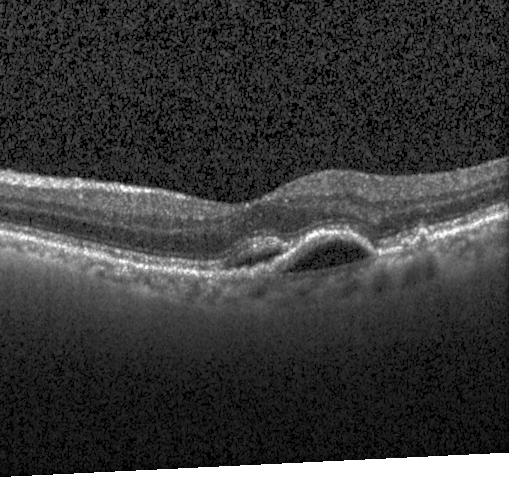

Spectral-domain OCT, Heidelberg Spectralis, fovea-centered, retinal OCT cross-section.
Finding: a choroidal neovascular membrane.